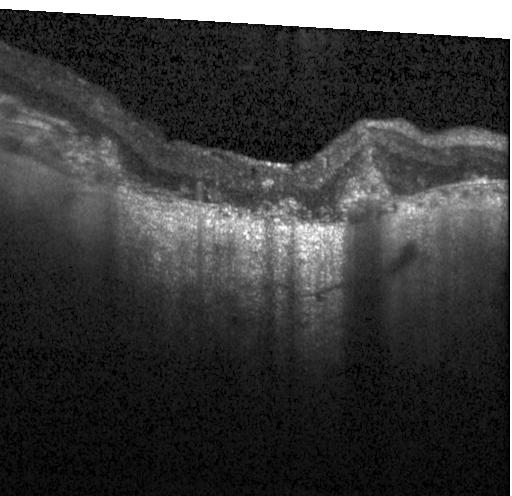
This B-scan demonstrates choroidal neovascularization.